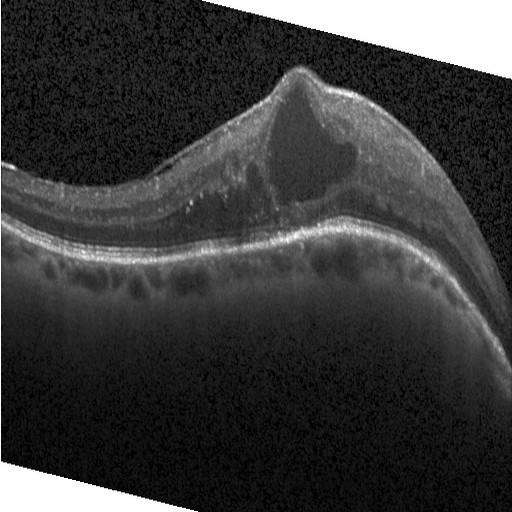 Through the macula, retinal OCT cross-section, instrument: Heidelberg Spectralis. The scan shows diabetic macular edema.